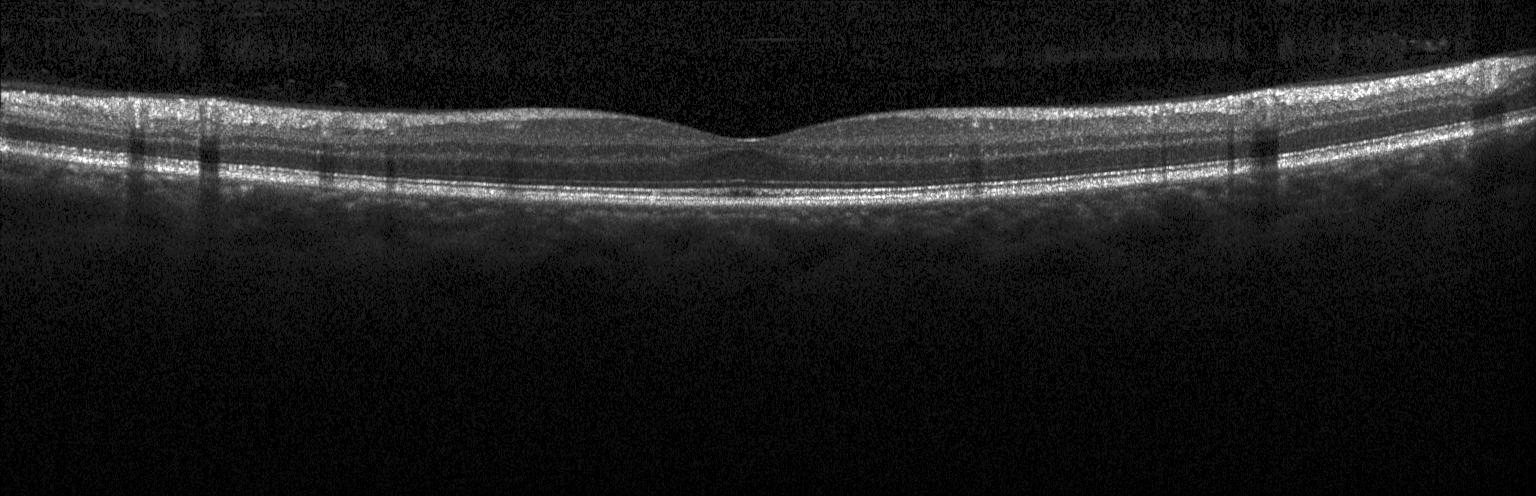
OCT B-scan — Diagnosis: no evidence of choroidal neovascularization, diabetic macular edema, or drusen.